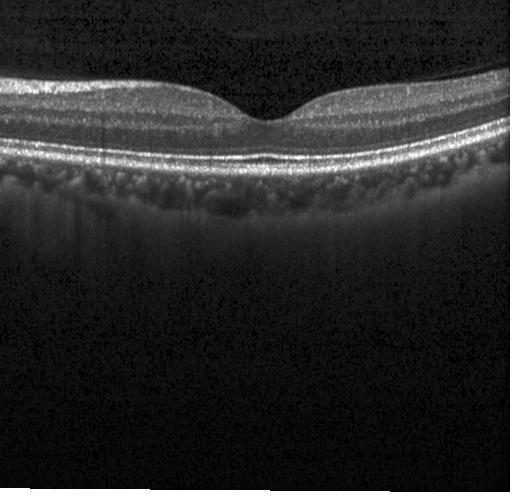
Heidelberg Spectralis OCT system. SD-OCT. Retinal OCT cross-section
This B-scan demonstrates no choroidal neovascularization, diabetic macular edema, or drusen.